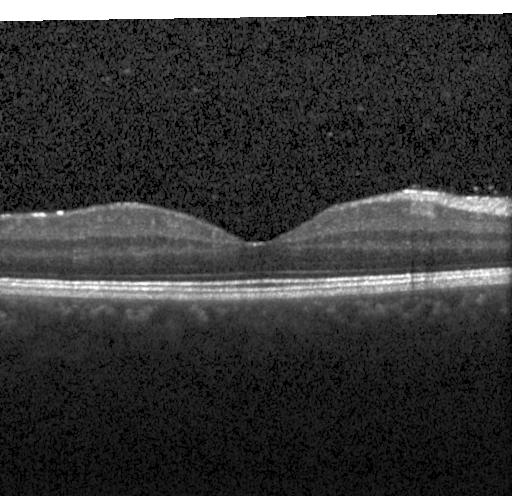
Diagnosis: no evidence of CNV, DME, or drusen.